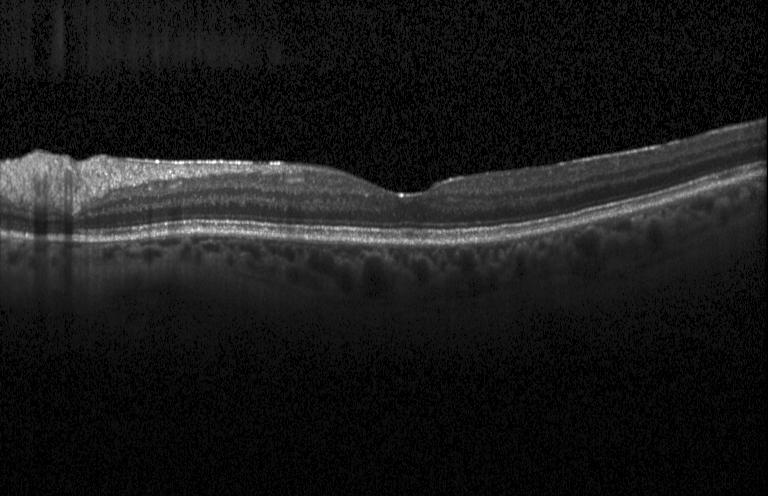

Instrument: Heidelberg Spectralis, through the macula, retinal OCT cross-section, SD-OCT. Macular OCT: no evidence of CNV, DME, or drusen.